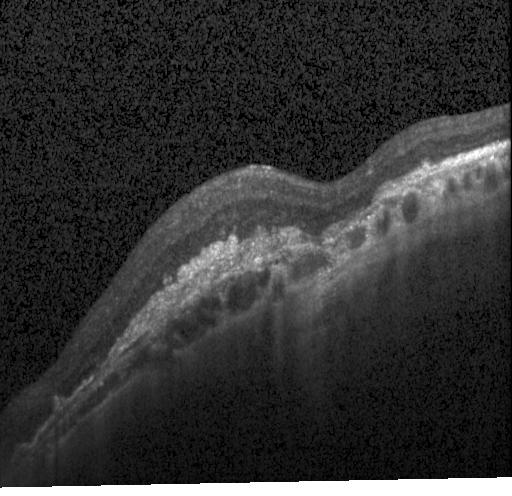

Fovea-centered. OCT line scan. Spectral-domain optical coherence tomography.
Assessment: a choroidal neovascular membrane.